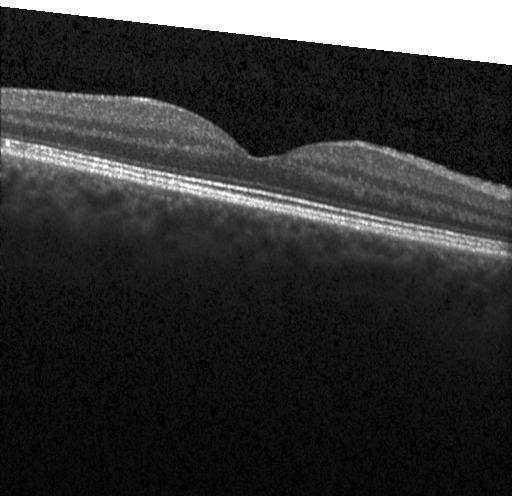

Macular scan. Acquired on a Heidelberg Spectralis. OCT B-scan. Finding: no choroidal neovascularization, diabetic macular edema, or drusen.